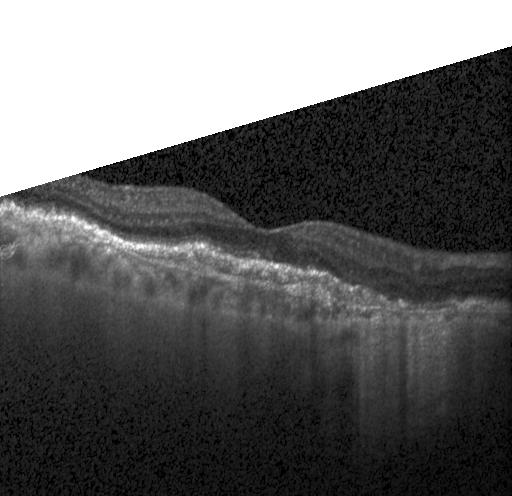

Acquired on a Heidelberg Spectralis; horizontal scan through the fovea; OCT B-scan — Macular OCT: a choroidal neovascular membrane.